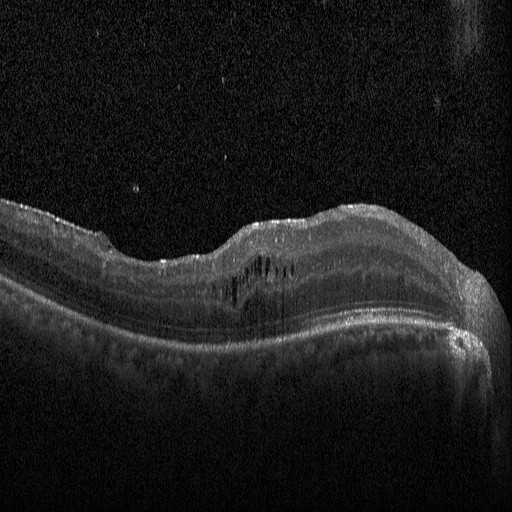 Heidelberg Spectralis OCT system. Retinal OCT cross-section. SD-OCT — The scan shows diabetic macular edema (DME).